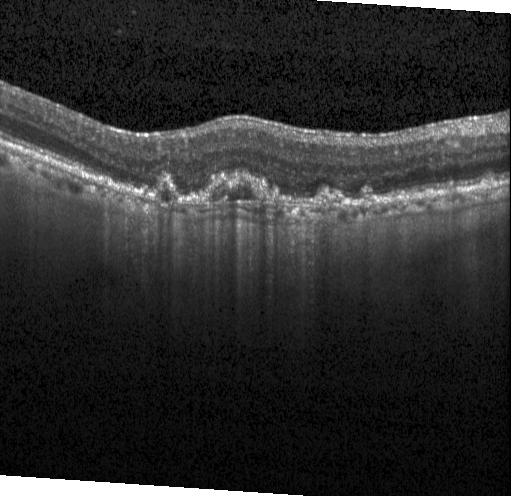 Diagnosis: a choroidal neovascular membrane.